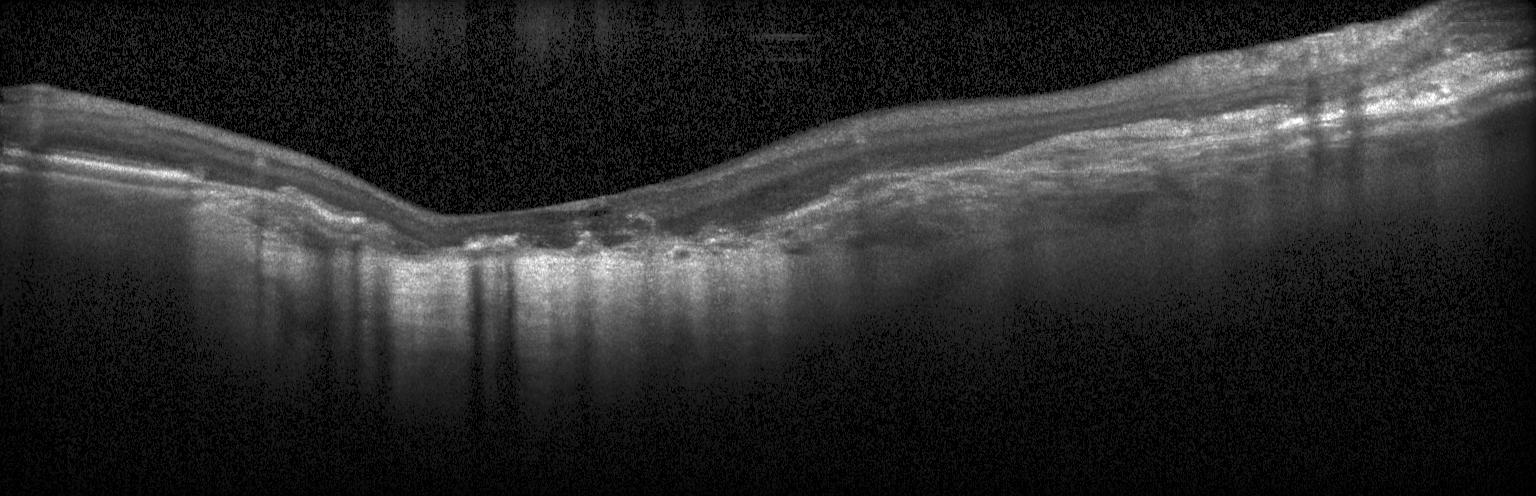

Macular OCT: a choroidal neovascular membrane.